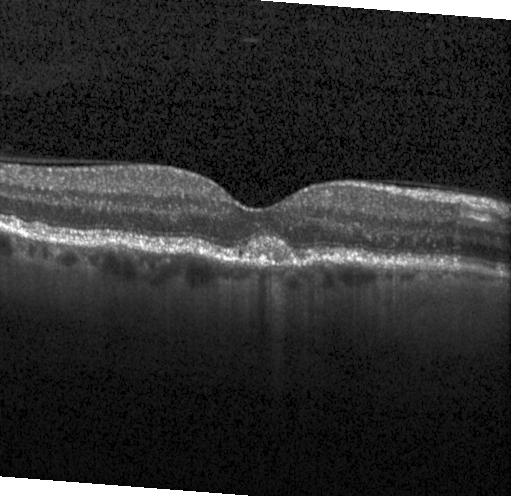

OCT B-scan
Diagnosis: drusen.